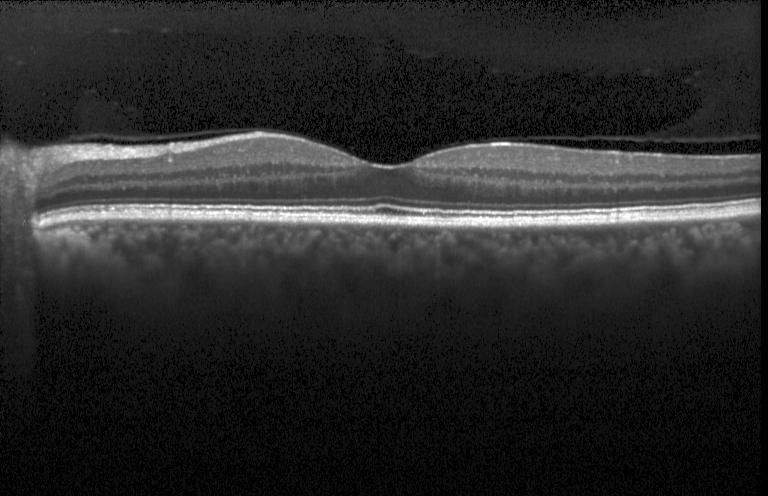 OCT finding: no choroidal neovascularization, no diabetic macular edema, and no drusen.